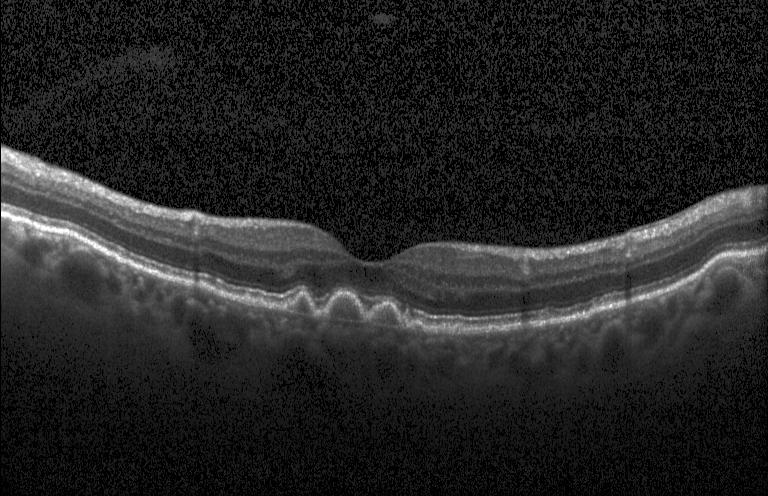
Acquired on a Heidelberg Spectralis. Macular scan. Retinal OCT cross-section — Assessment: multiple drusen.